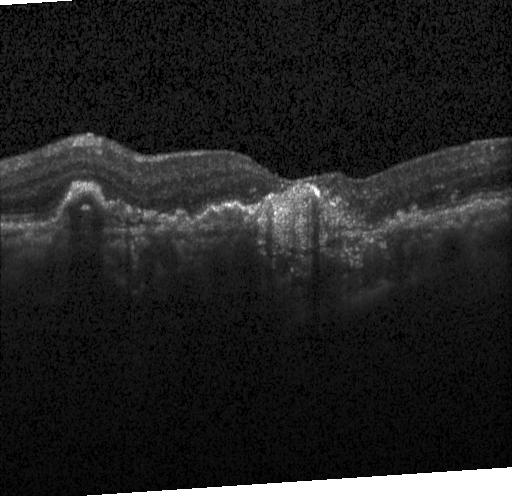

Heidelberg Spectralis OCT system, optical coherence tomography B-scan.
A choroidal neovascular membrane.